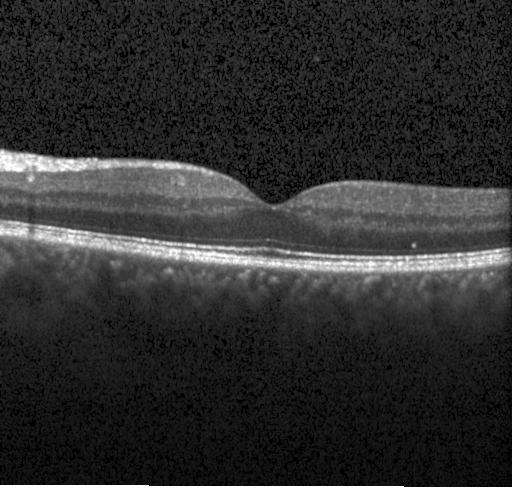
Macular OCT: neither CNV, DME, nor drusen.